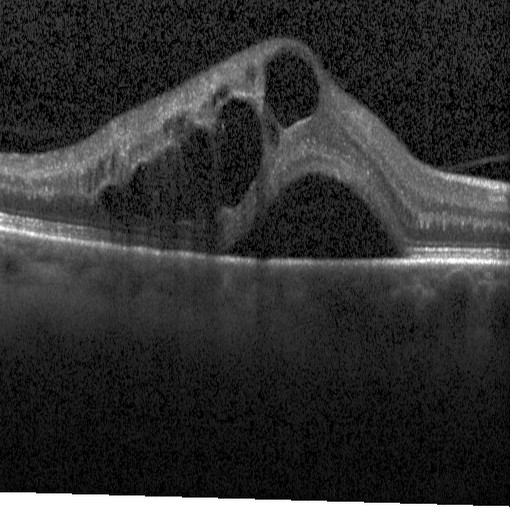 OCT line scan; centered on the fovea; Heidelberg Spectralis OCT system.
Finding: diabetic macular edema.